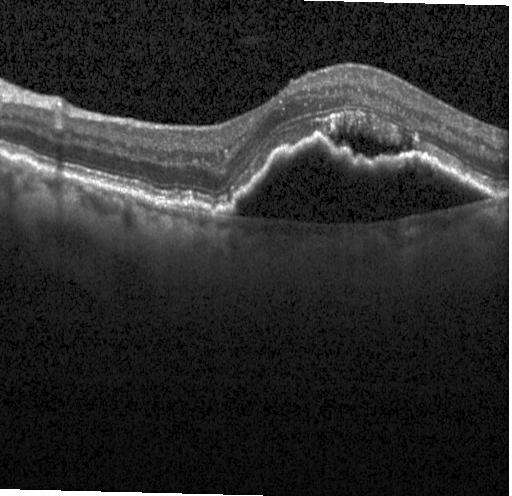

Acquired on a Heidelberg Spectralis. Retinal OCT B-scan.
CNV.